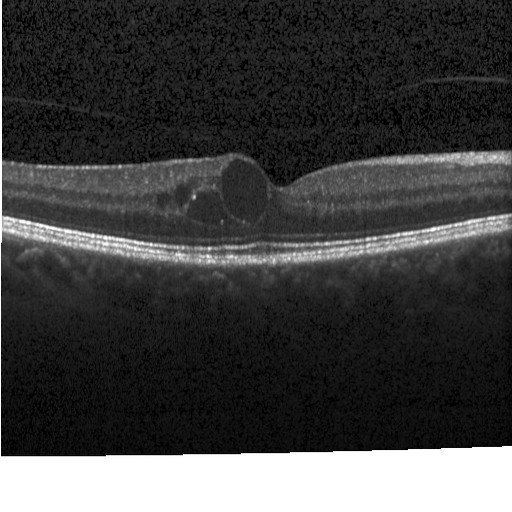

Spectral-domain OCT B-scan: diabetic macular edema (DME).